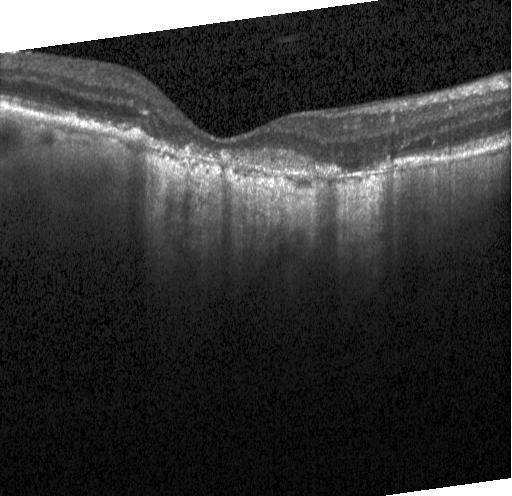 Fovea-centered · retinal OCT B-scan · Heidelberg Spectralis OCT system · spectral-domain OCT
This B-scan demonstrates choroidal neovascularization.